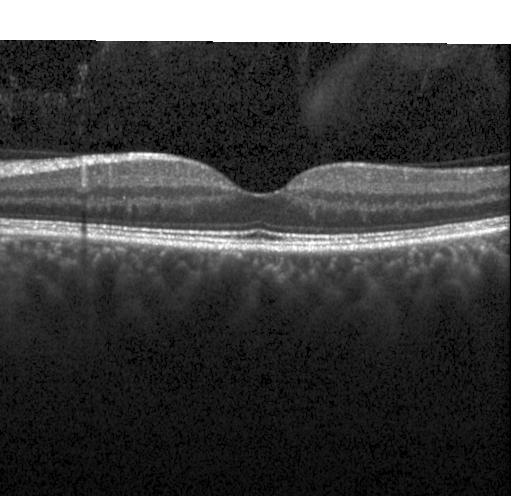
Retinal OCT cross-section showing neither choroidal neovascularization, diabetic macular edema, nor drusen.